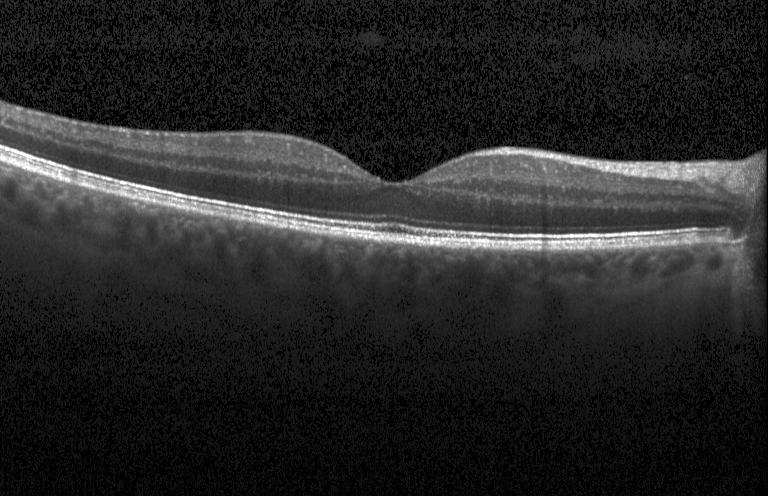 Macular OCT: no CNV, DME, or drusen.